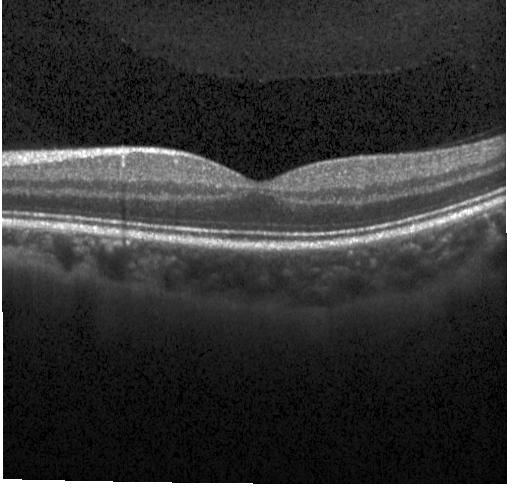

Optical coherence tomography B-scan — Impression: neither choroidal neovascularization, diabetic macular edema, nor drusen.